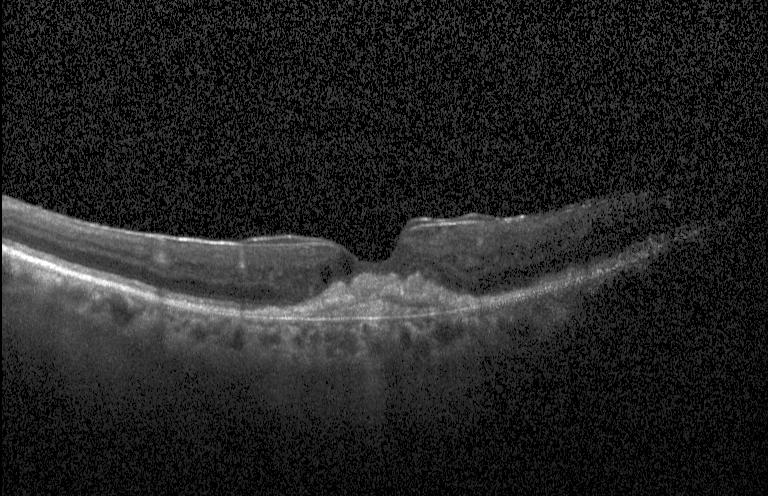

OCT scan showing a choroidal neovascular membrane.